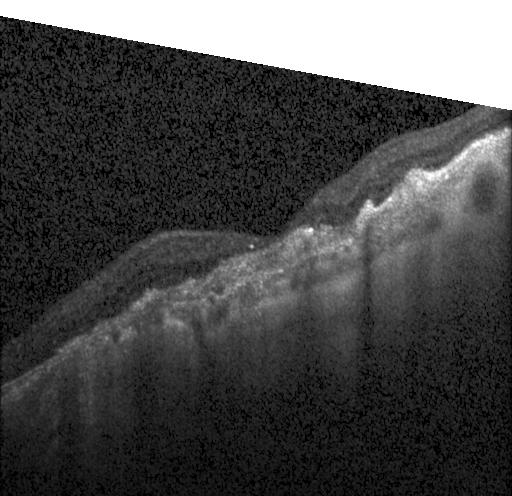
OCT B-scan showing choroidal neovascularization.